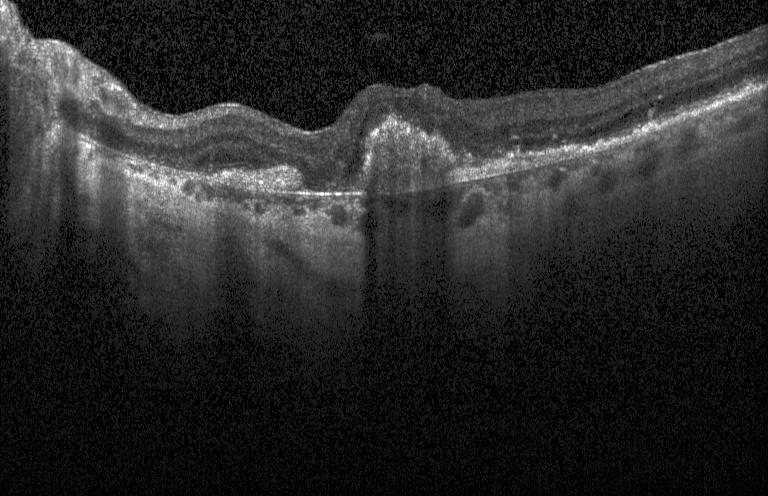

Optical coherence tomography scan · spectral-domain OCT · fovea-centered. This B-scan demonstrates a choroidal neovascular membrane.